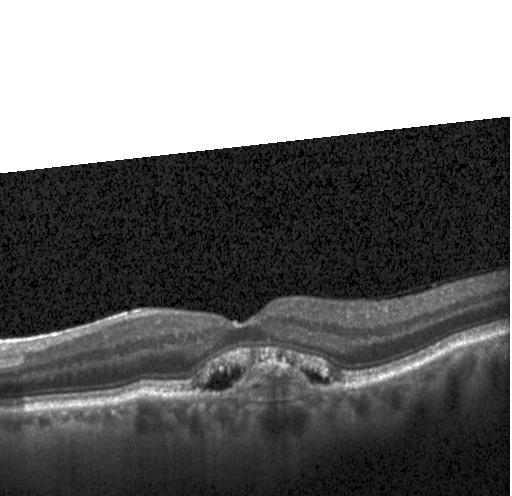
Spectral-domain optical coherence tomography. Heidelberg Spectralis. Retinal OCT cross-section — Macular OCT: a choroidal neovascular membrane.